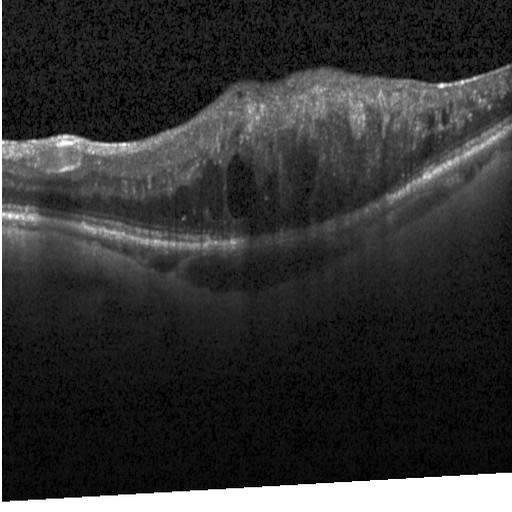

Retinal OCT cross-section. This B-scan demonstrates diabetic macular edema (DME).